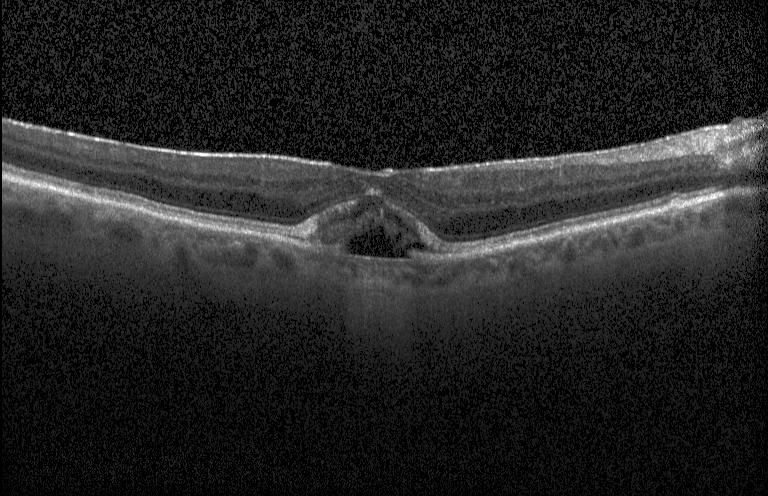
OCT B-scan. Macular OCT: CNV.